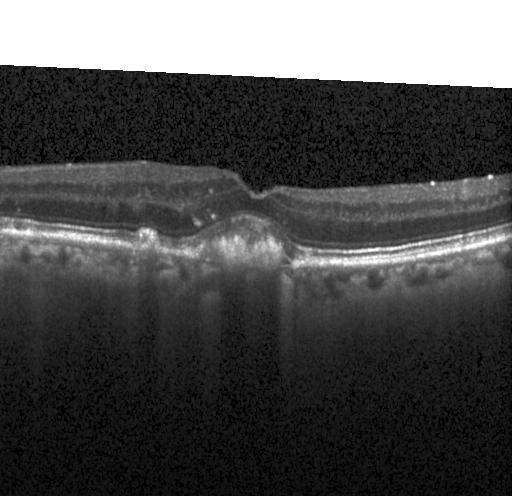

OCT B-scan.
Choroidal neovascularization (CNV).